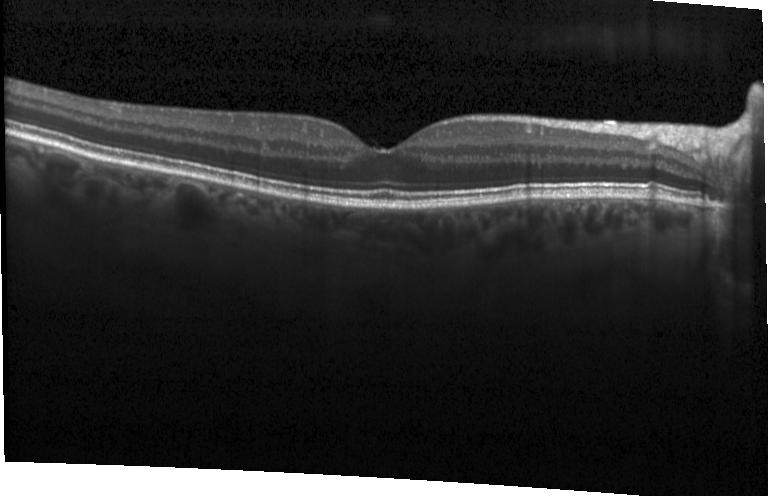
Spectral-domain OCT · OCT B-scan.
Finding: neither choroidal neovascularization, diabetic macular edema, nor drusen.